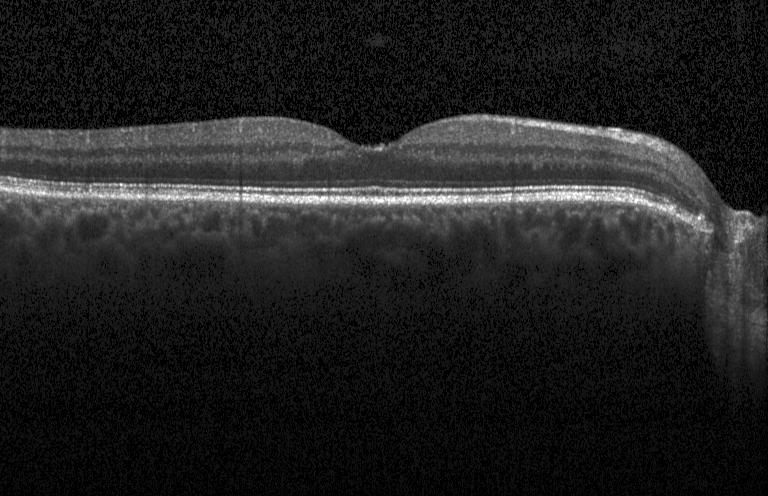

Retinal OCT cross-section. Instrument: Heidelberg Spectralis
Impression: no choroidal neovascularization, diabetic macular edema, or drusen.